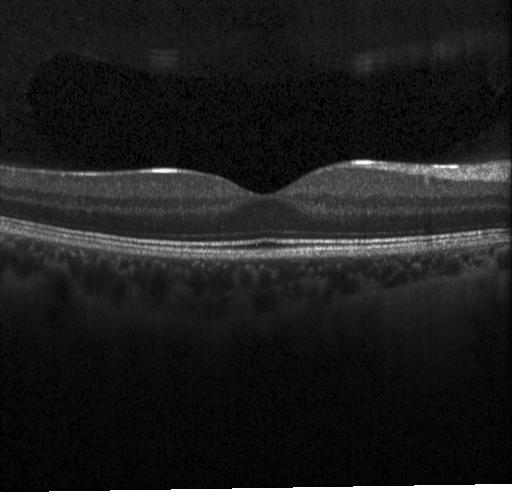 SD-OCT. Heidelberg Spectralis. Horizontal scan through the fovea. OCT B-scan.
Diagnosis: no choroidal neovascularization, diabetic macular edema, or drusen.